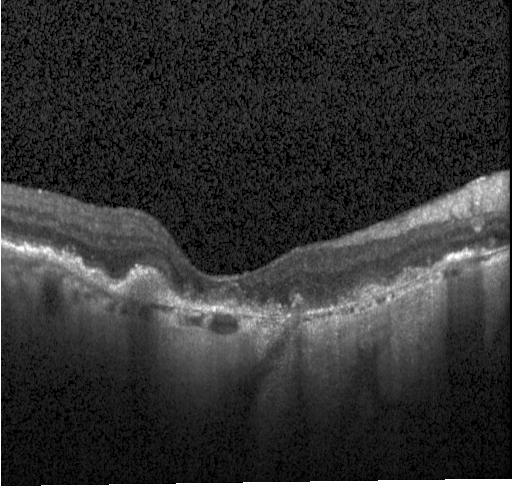

A choroidal neovascular membrane.